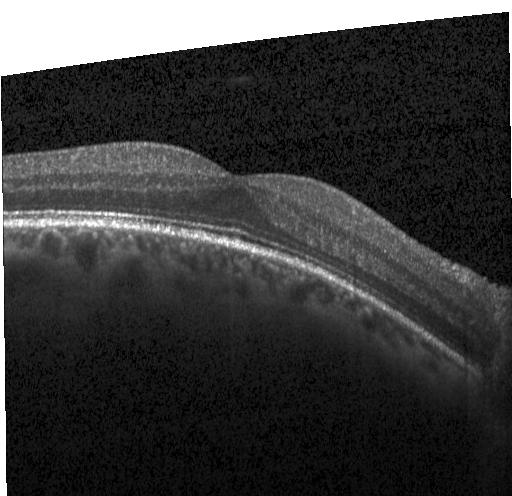

SD-OCT · OCT line scan · macular scan.
Impression: no evidence of choroidal neovascularization, diabetic macular edema, or drusen.